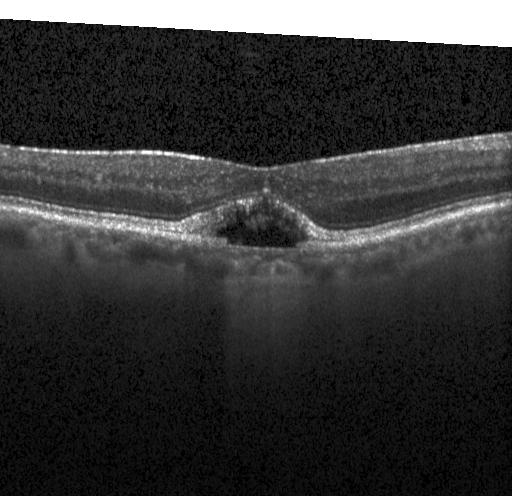

Optical coherence tomography scan — Finding: choroidal neovascularization.